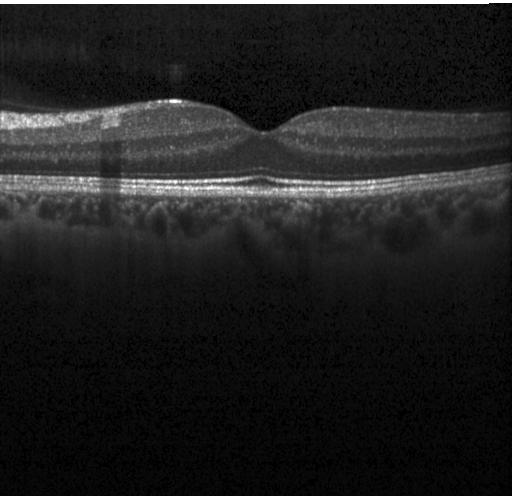 Retinal OCT B-scan.
Macular OCT: no evidence of choroidal neovascularization, diabetic macular edema, or drusen.